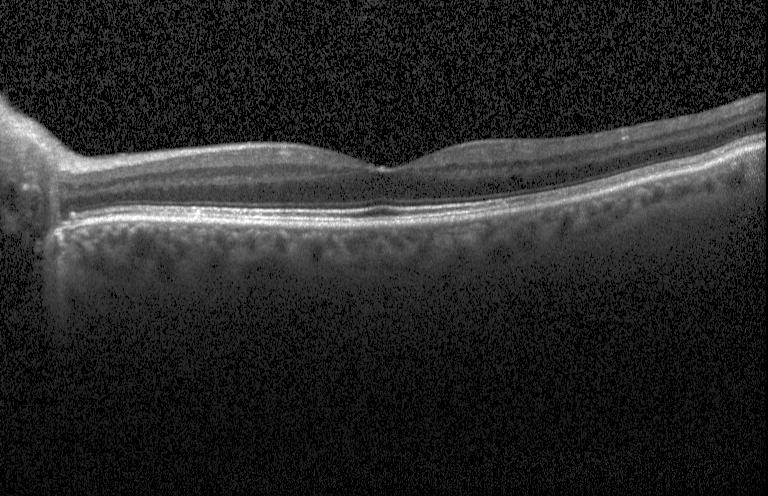 Impression: neither CNV, DME, nor drusen.